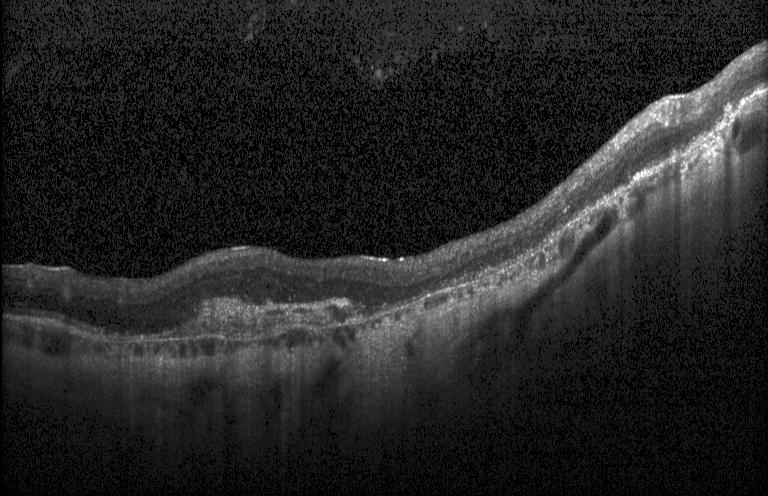

OCT finding: a choroidal neovascular membrane.